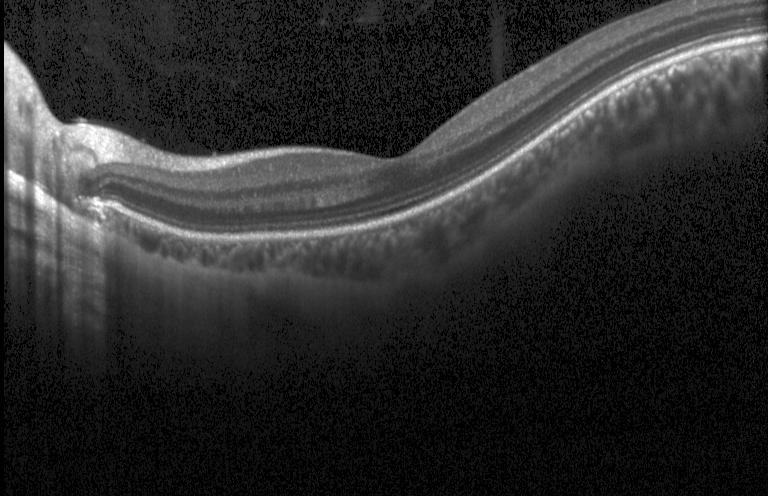
Macular OCT demonstrating no choroidal neovascularization, no diabetic macular edema, and no drusen.